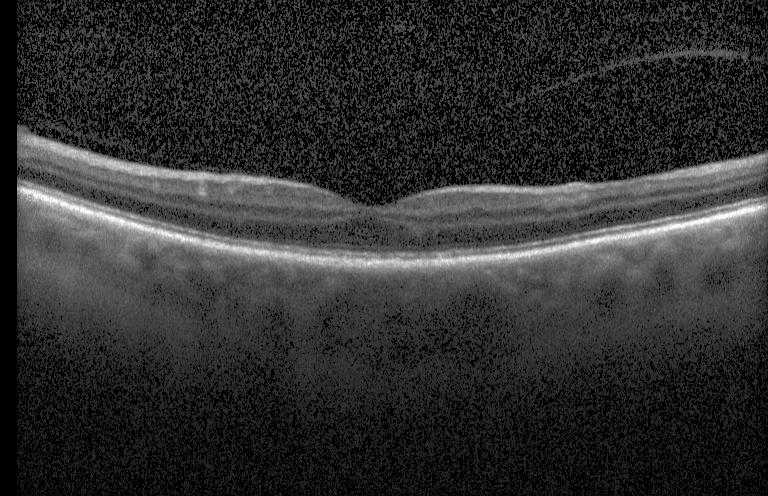
Spectral-domain optical coherence tomography, optical coherence tomography scan, acquired on a Heidelberg Spectralis. Impression: neither choroidal neovascularization, diabetic macular edema, nor drusen.